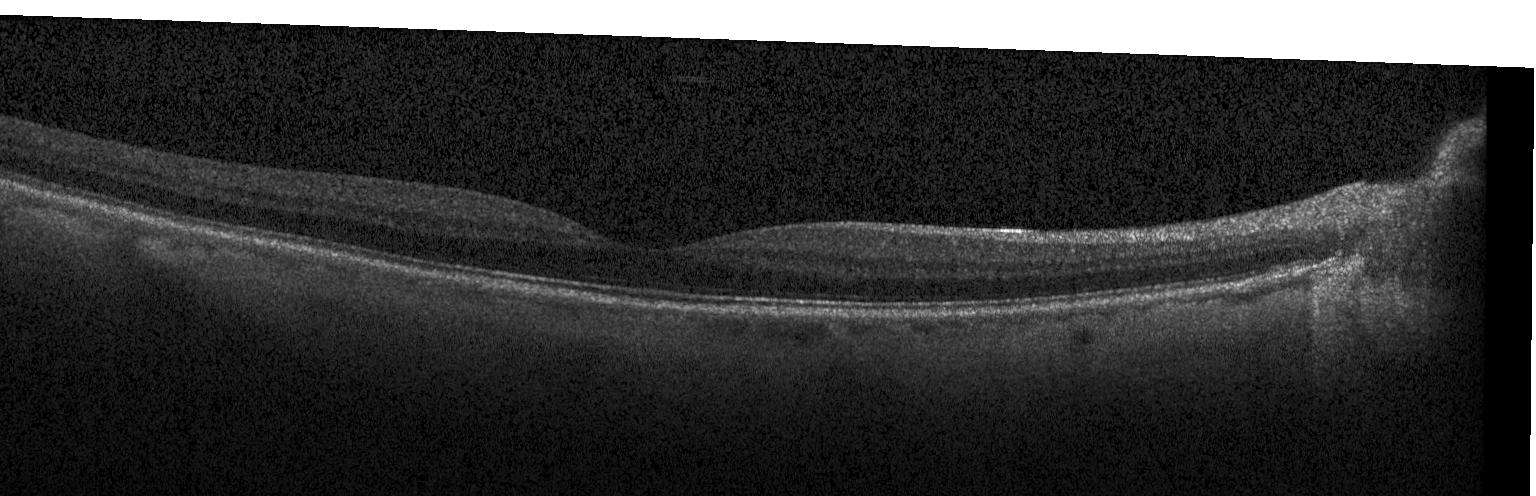
Heidelberg Spectralis OCT system, OCT line scan. Finding: no choroidal neovascularization, no diabetic macular edema, and no drusen.